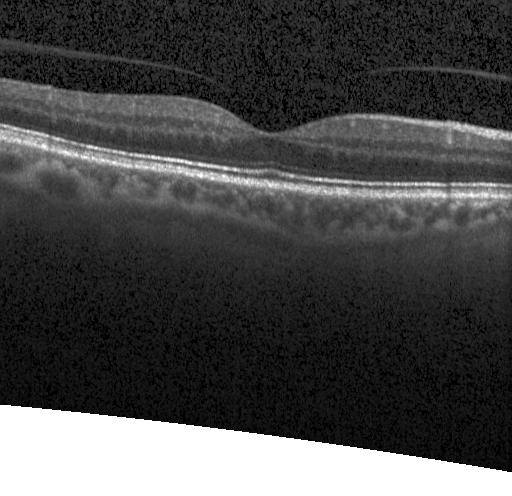 OCT finding: no choroidal neovascularization, no diabetic macular edema, and no drusen.